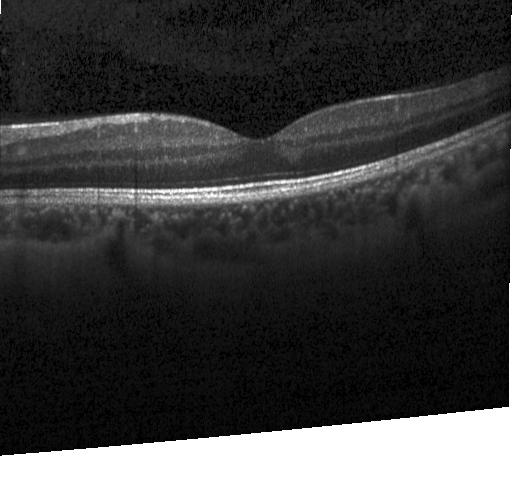 OCT finding: no CNV, no DME, and no drusen.